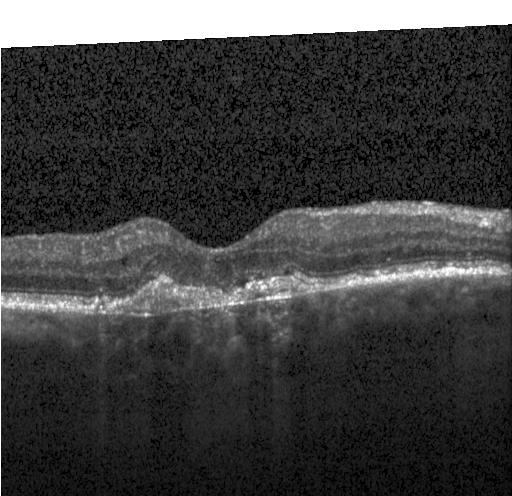 OCT line scan · spectral-domain optical coherence tomography · acquired on a Heidelberg Spectralis · horizontal scan through the fovea — A choroidal neovascular membrane.